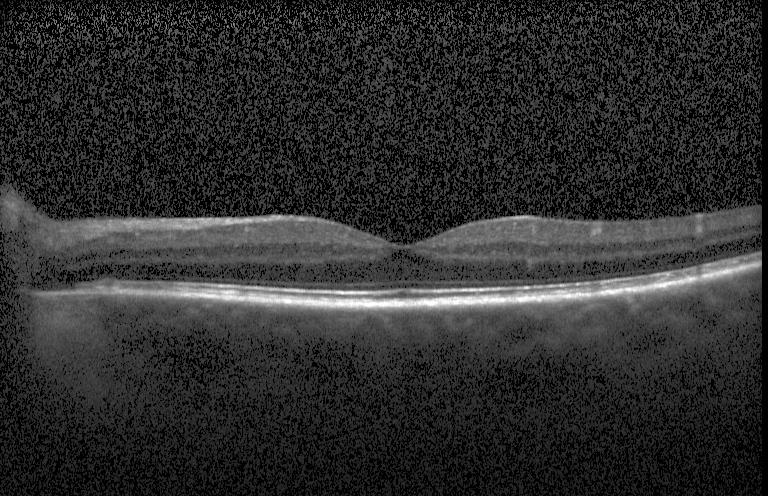 Macular scan; spectral-domain optical coherence tomography; Heidelberg Spectralis OCT system; retinal OCT B-scan. Assessment: no evidence of CNV, DME, or drusen.